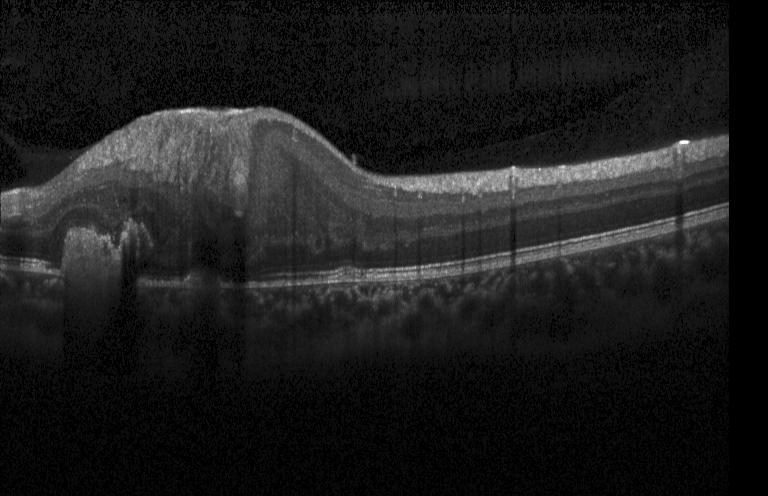 Retinal OCT cross-section, spectral-domain OCT, fovea-centered, Heidelberg Spectralis — Diagnosis: a choroidal neovascular membrane.